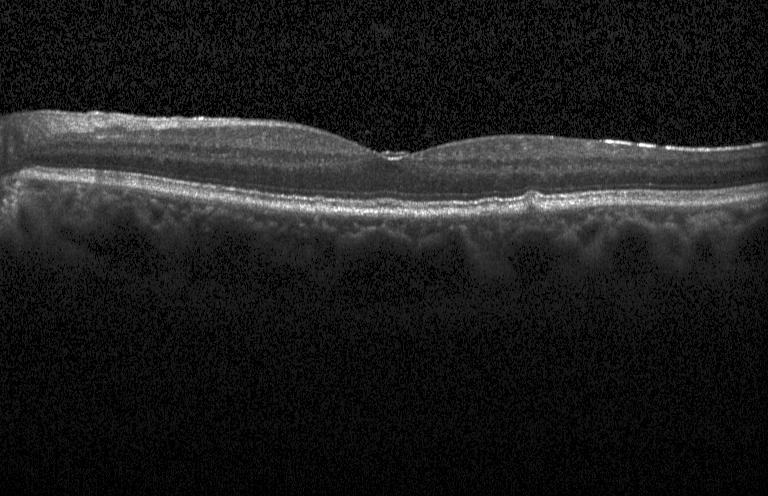
Instrument: Heidelberg Spectralis; macular scan; OCT line scan. Finding: multiple drusen.